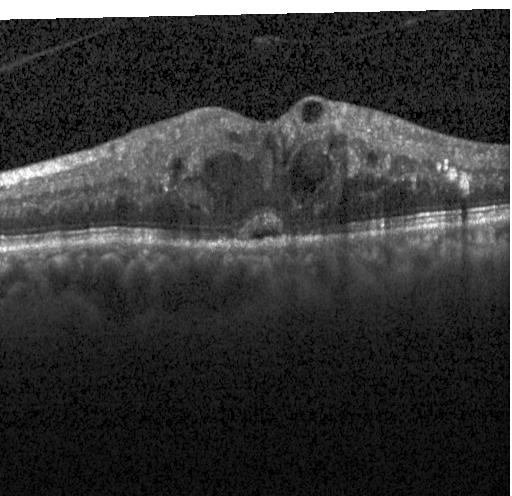

Retinal OCT cross-section — Dx: diabetic macular edema (DME).